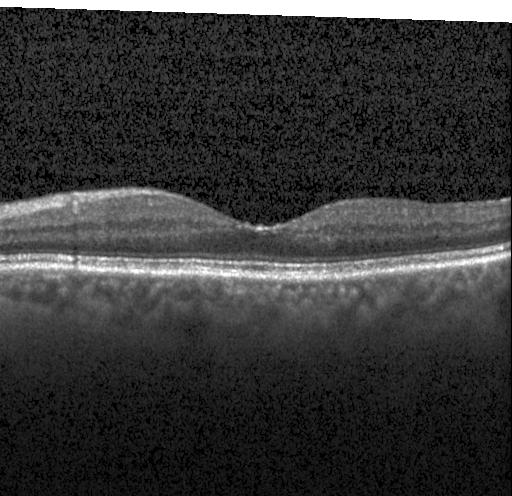

Finding: no CNV, DME, or drusen.